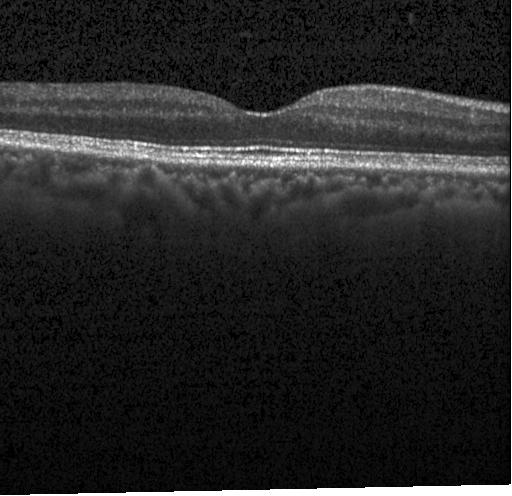

OCT B-scan.
Diagnosis: no choroidal neovascularization, no diabetic macular edema, and no drusen.